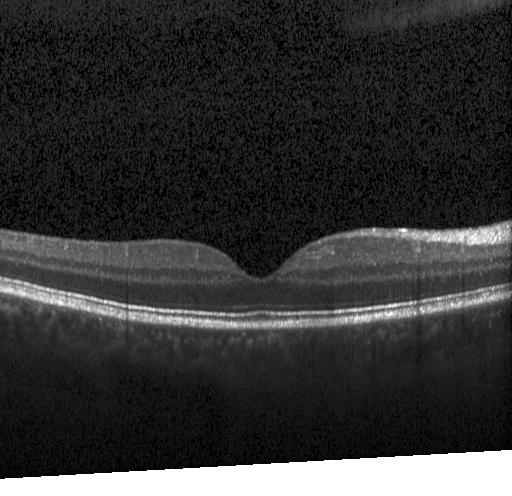 Centered on the fovea; acquired on a Heidelberg Spectralis; OCT line scan.
OCT finding: no choroidal neovascularization, diabetic macular edema, or drusen.